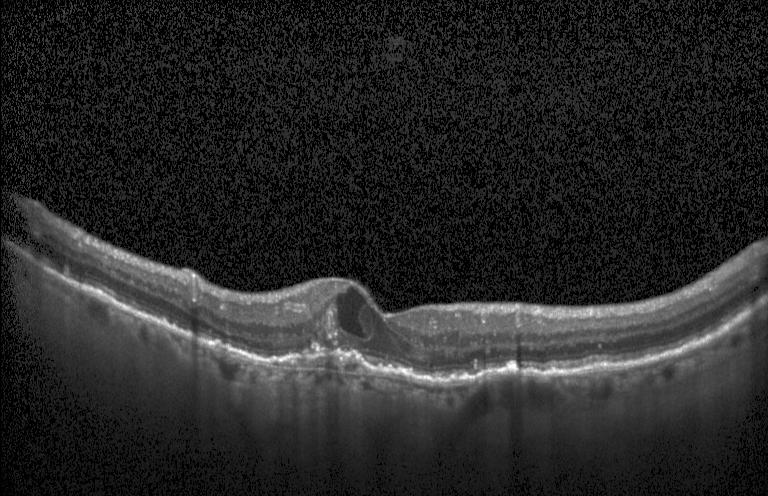

Retinal OCT cross-section.
This B-scan demonstrates CNV.